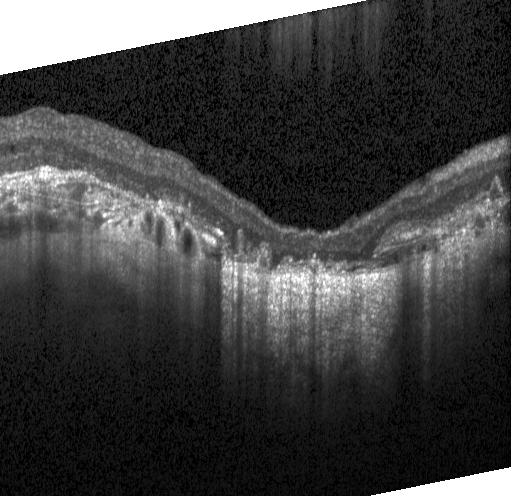 Optical coherence tomography B-scan · macular scan.
OCT finding: choroidal neovascularization (CNV).